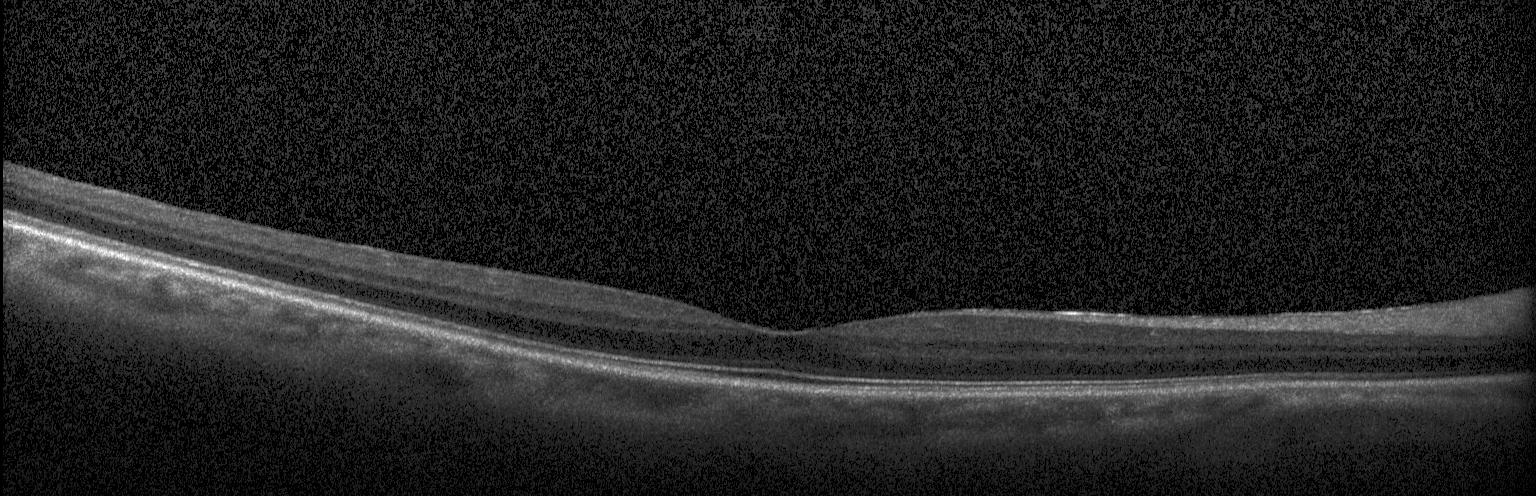

Macular scan · OCT B-scan · SD-OCT · Heidelberg Spectralis OCT system — Assessment: no choroidal neovascularization, diabetic macular edema, or drusen.